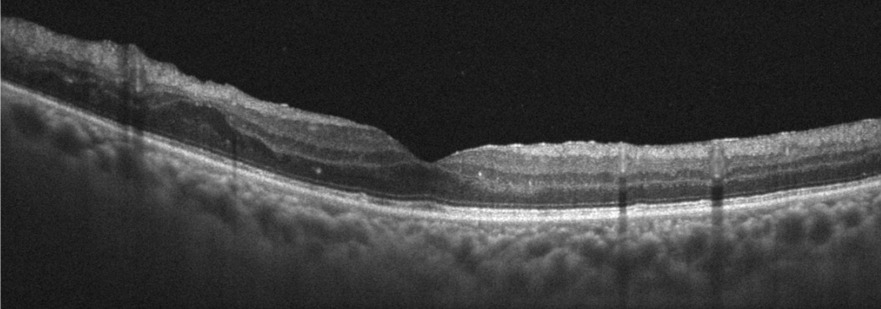 Fovea-centered; OCT line scan; Optovue Avanti RTVue XR.
Finding: DME.